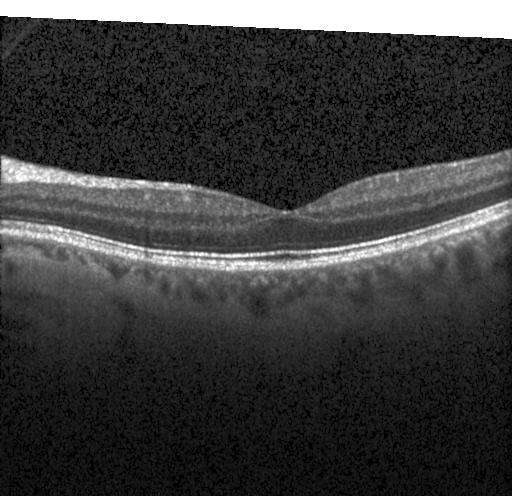 Acquired on a Heidelberg Spectralis · retinal OCT B-scan · macular scan
Assessment: no CNV, DME, or drusen.